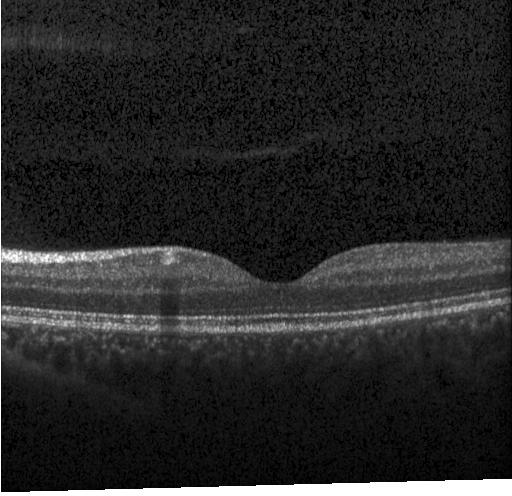 OCT line scan, Heidelberg Spectralis.
Finding: no evidence of choroidal neovascularization, diabetic macular edema, or drusen.